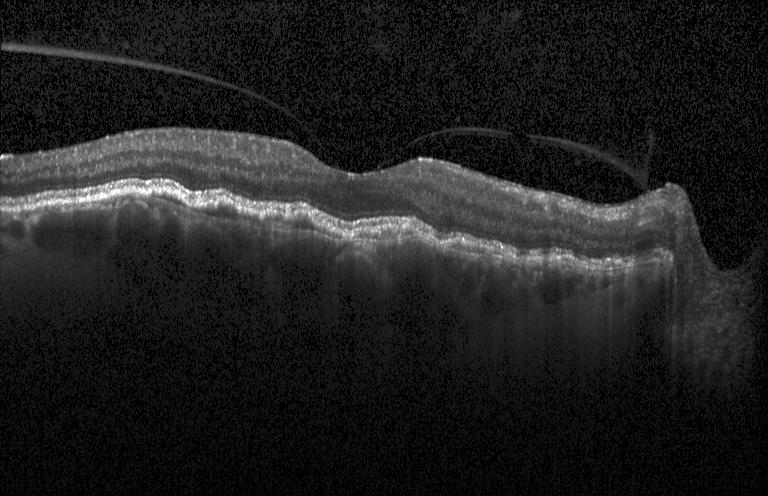 Optical coherence tomography scan; Heidelberg Spectralis — Diagnosis: CNV.